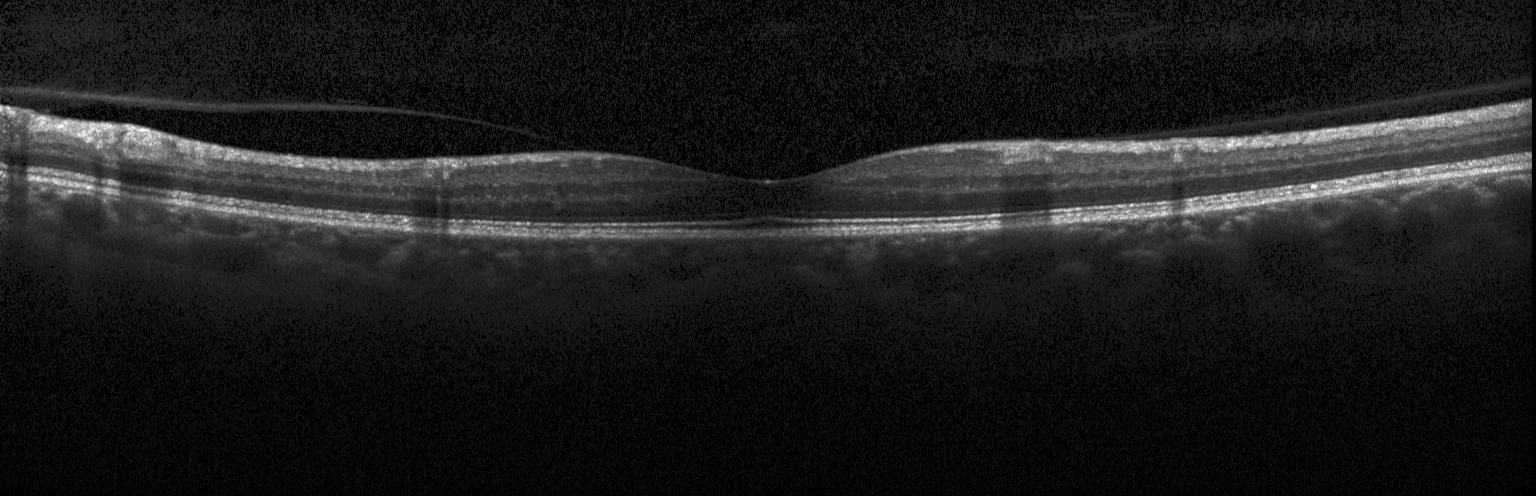 Optical coherence tomography scan. Macular OCT: no choroidal neovascularization, diabetic macular edema, or drusen.